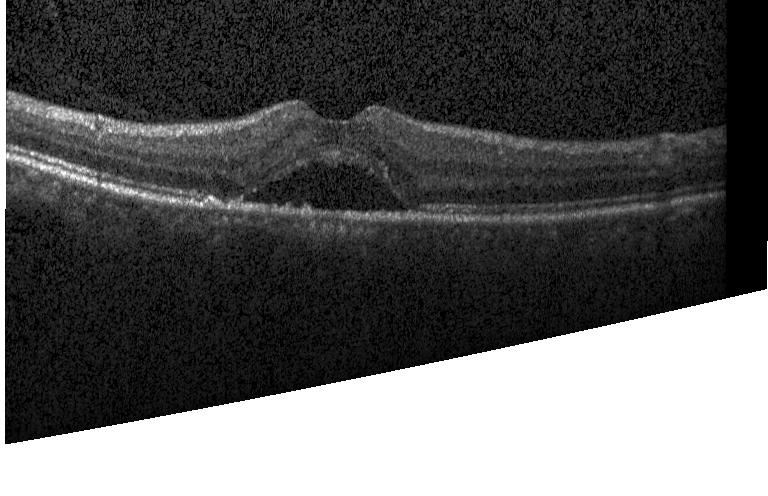
Assessment: a choroidal neovascular membrane.